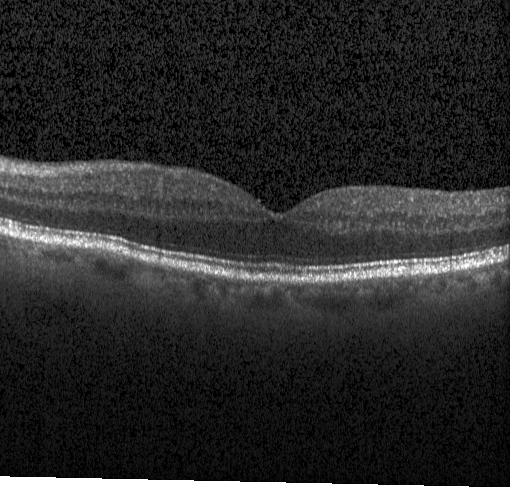

Diagnosis: neither CNV, DME, nor drusen.